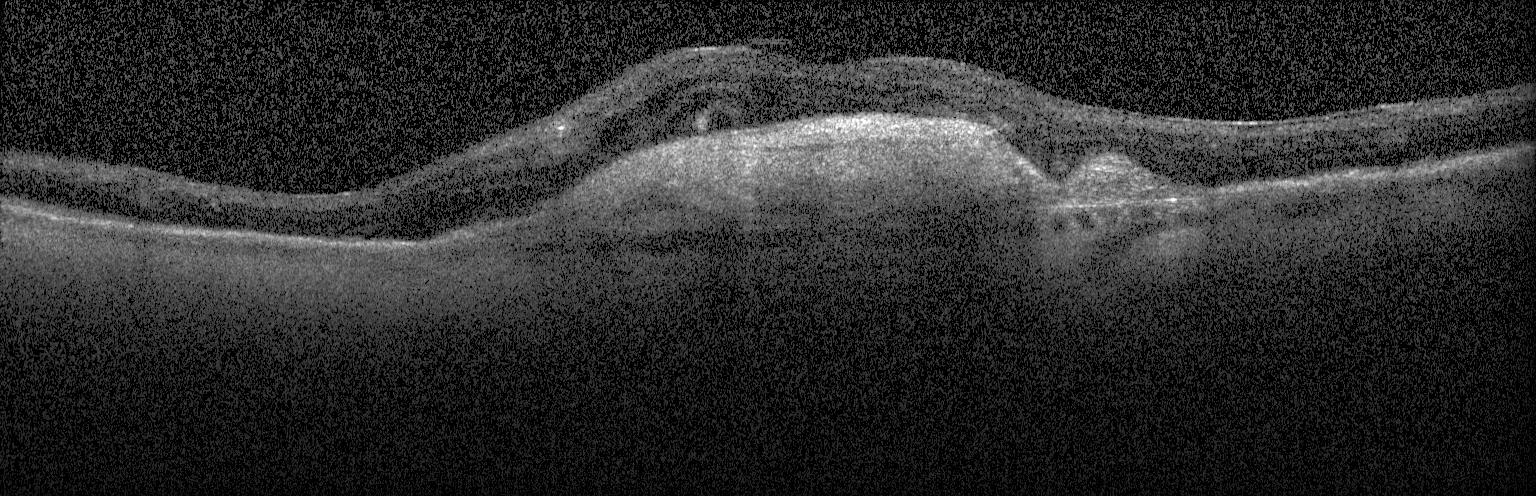 SD-OCT, OCT B-scan — Finding: choroidal neovascularization.